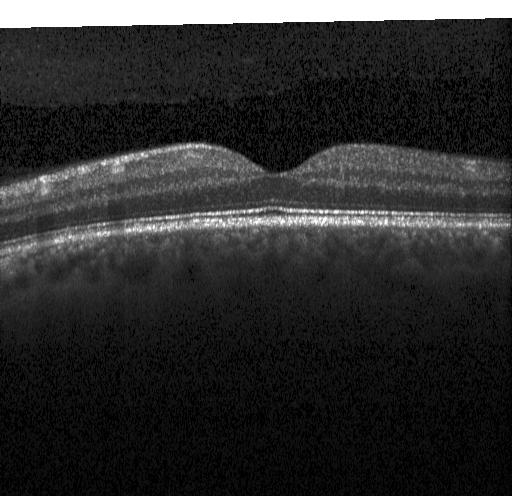
SD-OCT. OCT B-scan.
Finding: no choroidal neovascularization, no diabetic macular edema, and no drusen.